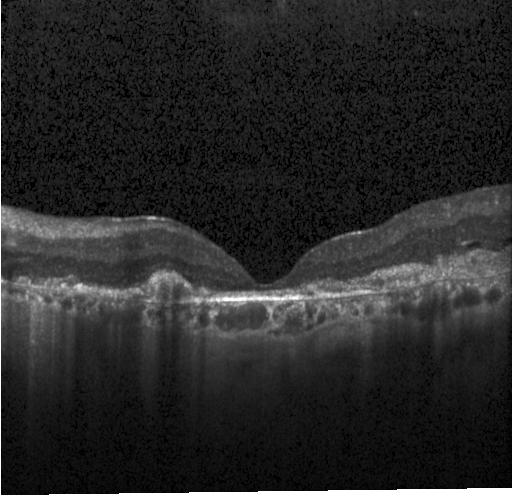 Macular OCT: choroidal neovascularization.